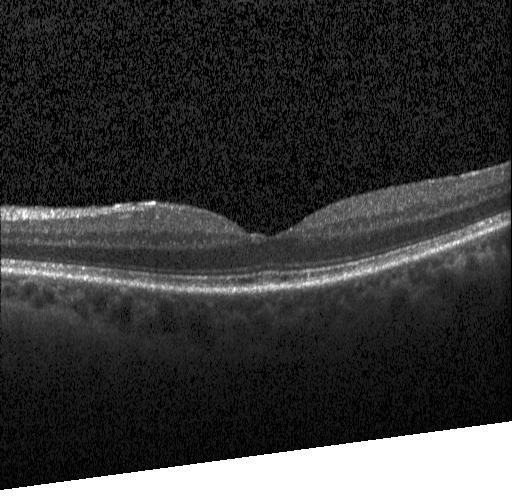 Retinal OCT B-scan, acquired on a Heidelberg Spectralis, SD-OCT. OCT finding: no CNV, no DME, and no drusen.